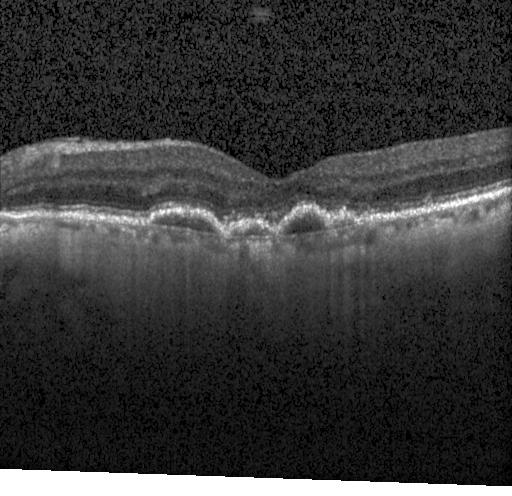
OCT scan showing CNV.